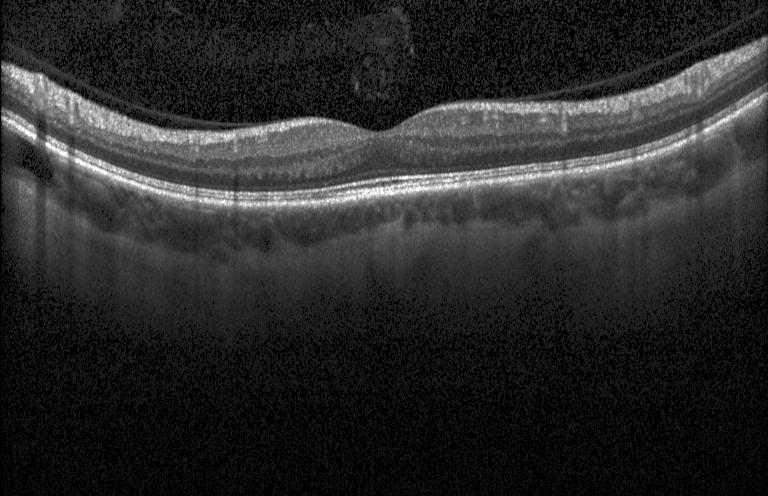 Retinal OCT B-scan. No choroidal neovascularization, no diabetic macular edema, and no drusen.